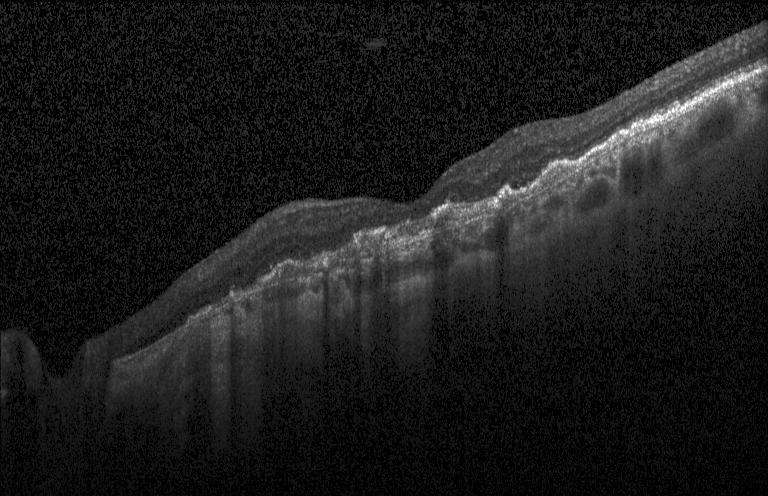 Diagnosis: choroidal neovascularization.